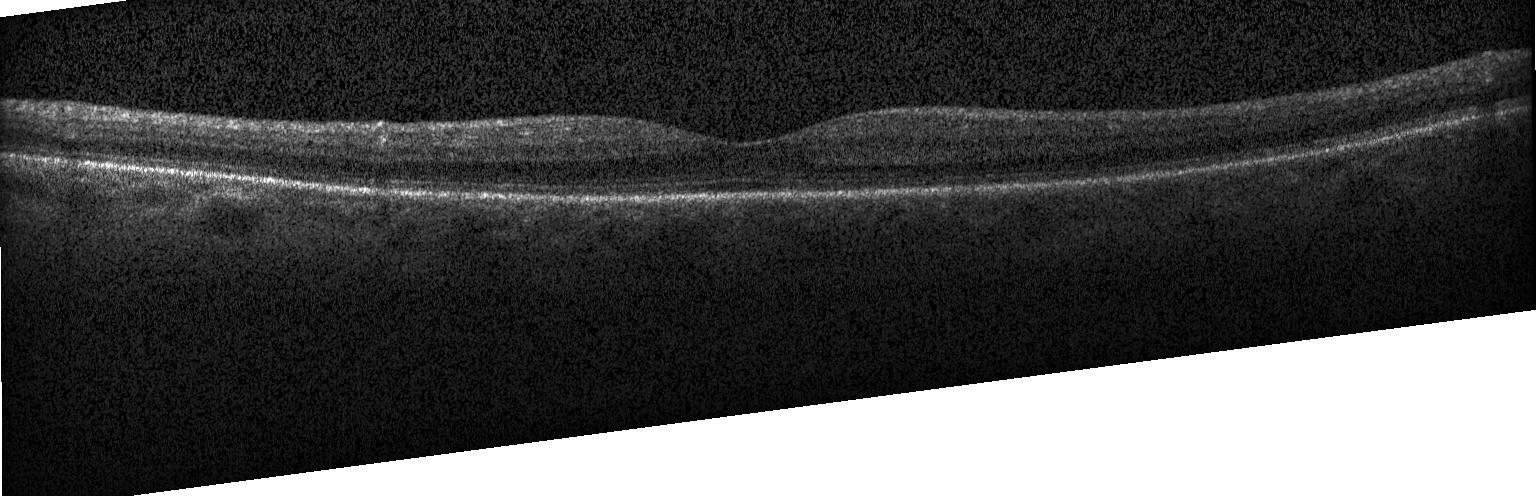 Spectral-domain OCT B-scan: no choroidal neovascularization, diabetic macular edema, or drusen.